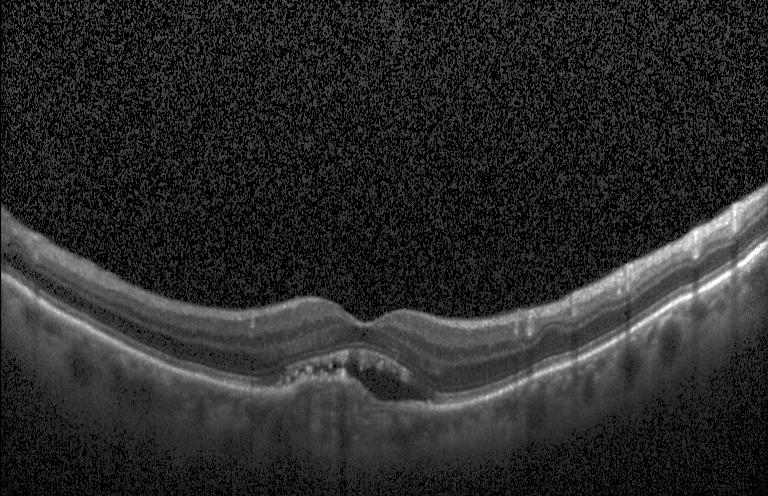
Retinal OCT B-scan · SD-OCT — Diagnosis: CNV.